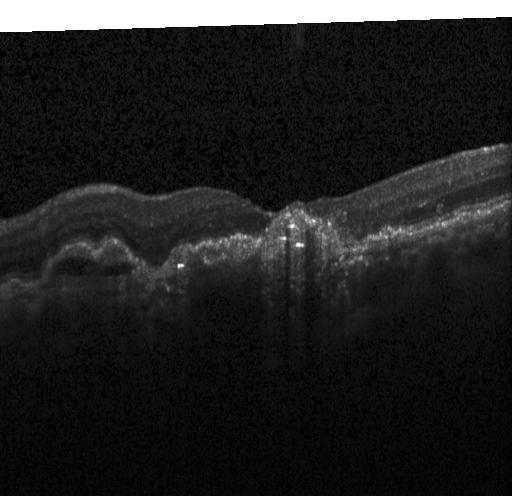
Retinal OCT B-scan. Through the macula. Heidelberg Spectralis OCT system. This B-scan demonstrates CNV.